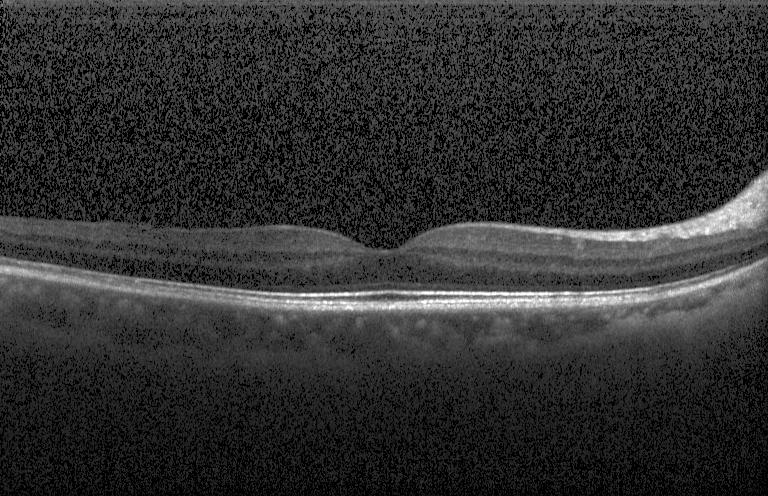 OCT finding: no choroidal neovascularization, no diabetic macular edema, and no drusen.